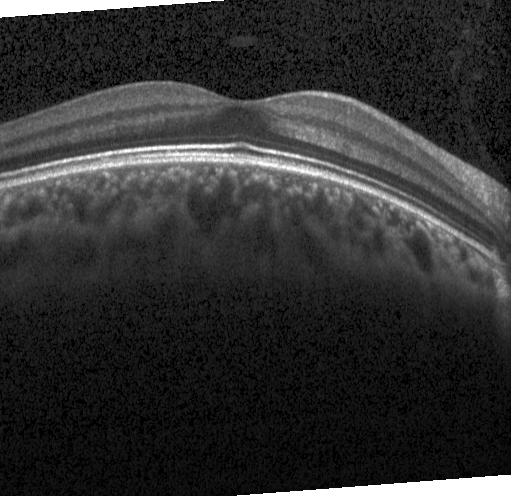
Retinal OCT cross-section — Dx: no choroidal neovascularization, no diabetic macular edema, and no drusen.